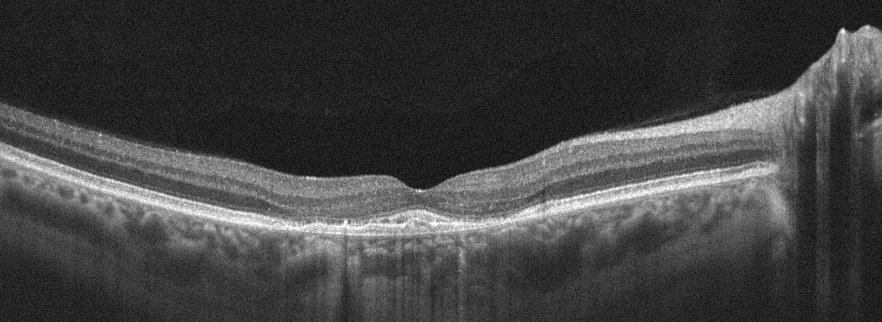

Right eye, optical coherence tomography B-scan — The scan shows AMD.